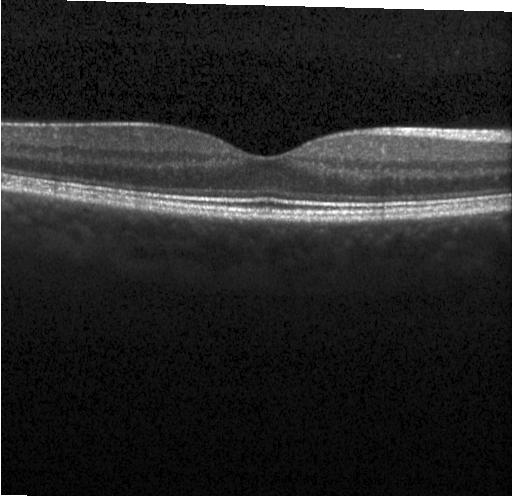
Assessment: neither CNV, DME, nor drusen.